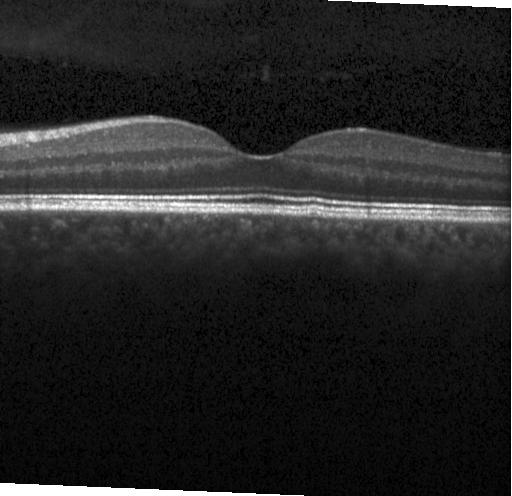

OCT finding: no evidence of choroidal neovascularization, diabetic macular edema, or drusen.